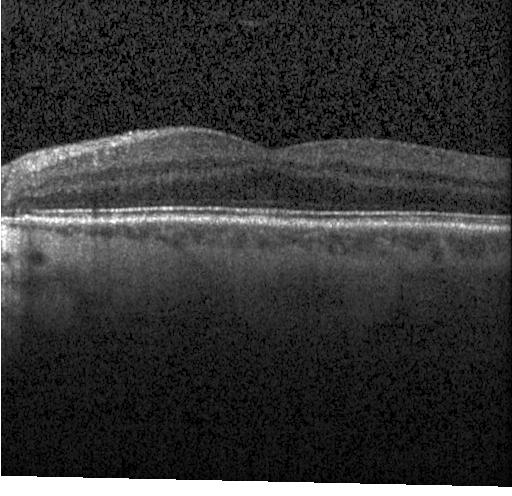

Centered on the fovea, acquired on a Heidelberg Spectralis, retinal OCT cross-section — Impression: no evidence of CNV, DME, or drusen.